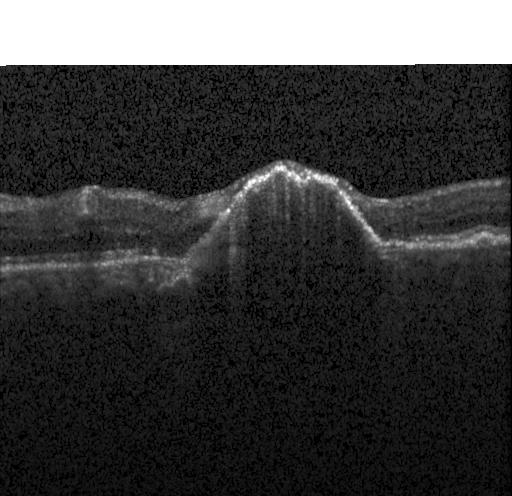
Optical coherence tomography B-scan.
The scan shows a choroidal neovascular membrane.